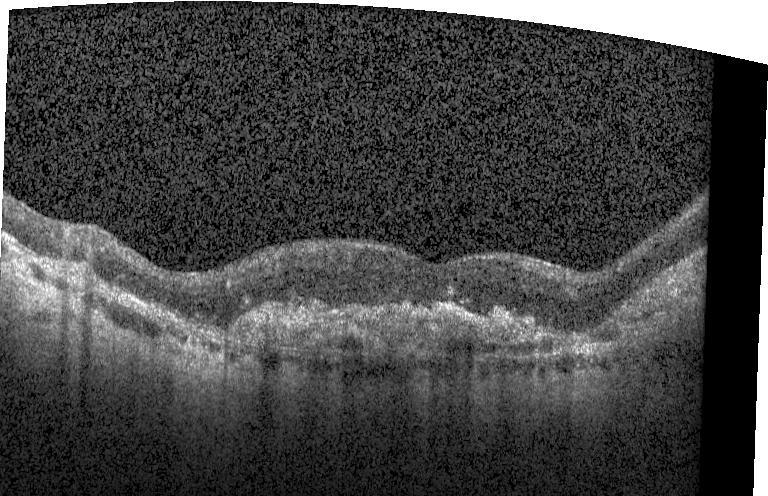
Heidelberg Spectralis OCT system, optical coherence tomography scan
Assessment: a choroidal neovascular membrane.